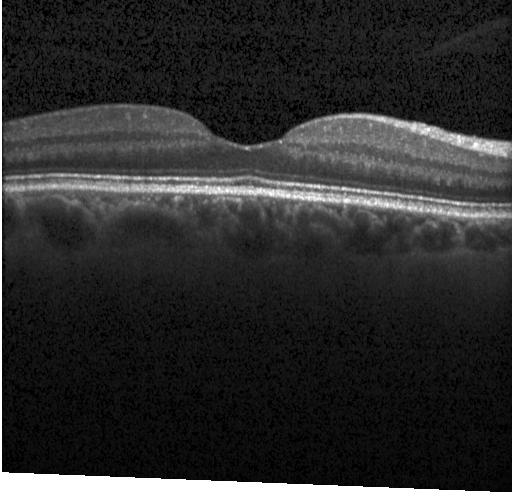
Impression: no CNV, no DME, and no drusen.